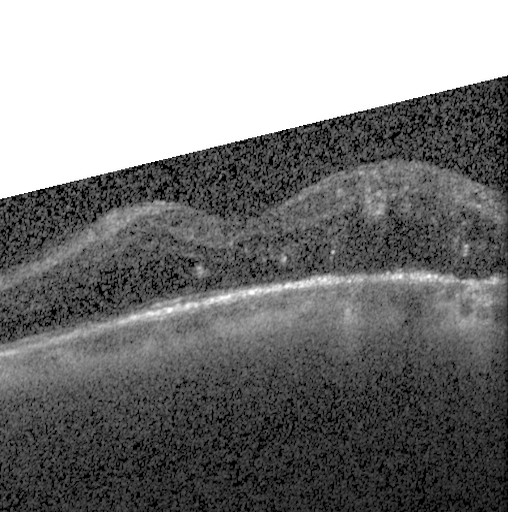 Impression: DME.